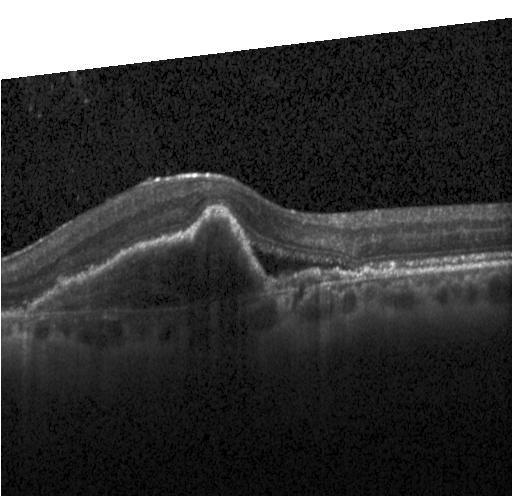 Spectral-domain OCT B-scan: CNV.